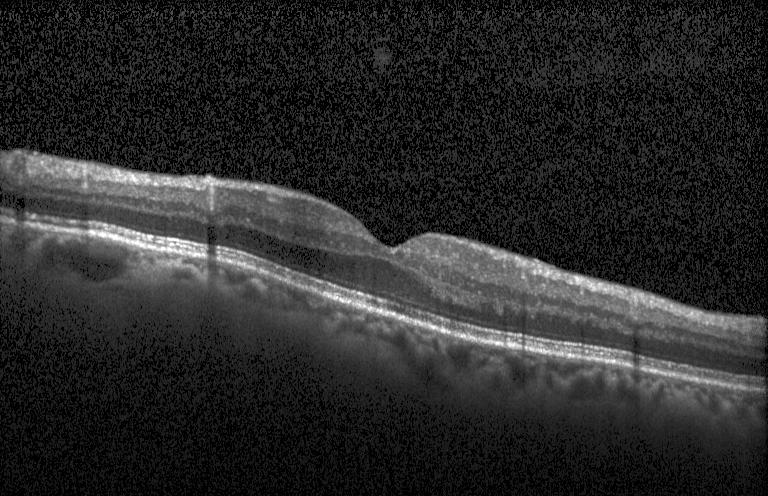 Dx: no evidence of choroidal neovascularization, diabetic macular edema, or drusen.